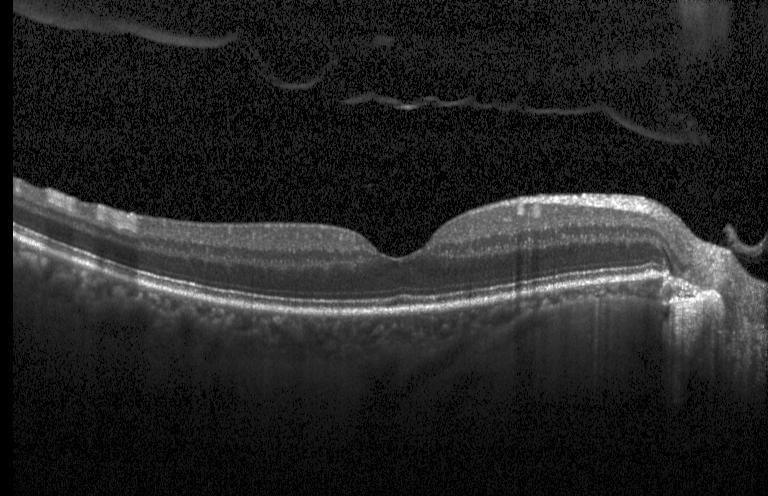
OCT B-scan; instrument: Heidelberg Spectralis.
Dx: no CNV, no DME, and no drusen.